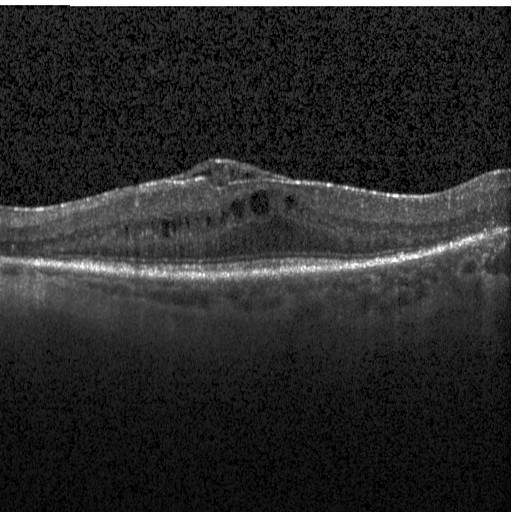
Optical coherence tomography B-scan.
Finding: diabetic macular edema.